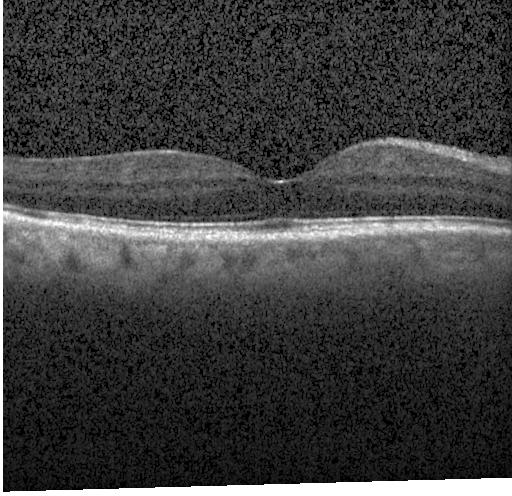

Finding: no evidence of CNV, DME, or drusen.